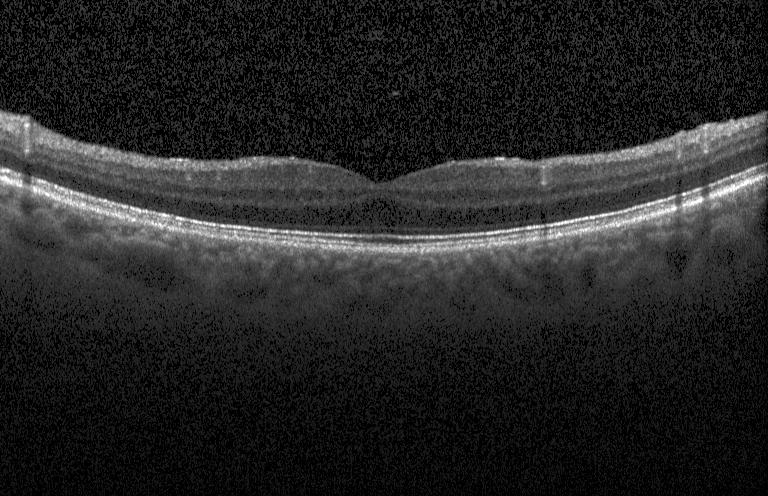

Optical coherence tomography scan
No evidence of choroidal neovascularization, diabetic macular edema, or drusen.